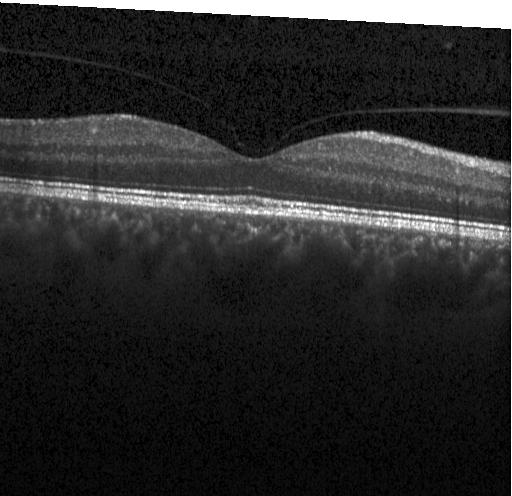 Macular OCT: no choroidal neovascularization, diabetic macular edema, or drusen.